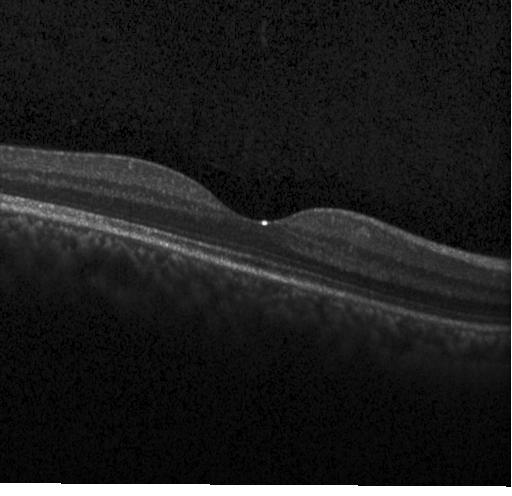
Optical coherence tomography scan
Dx: neither choroidal neovascularization, diabetic macular edema, nor drusen.